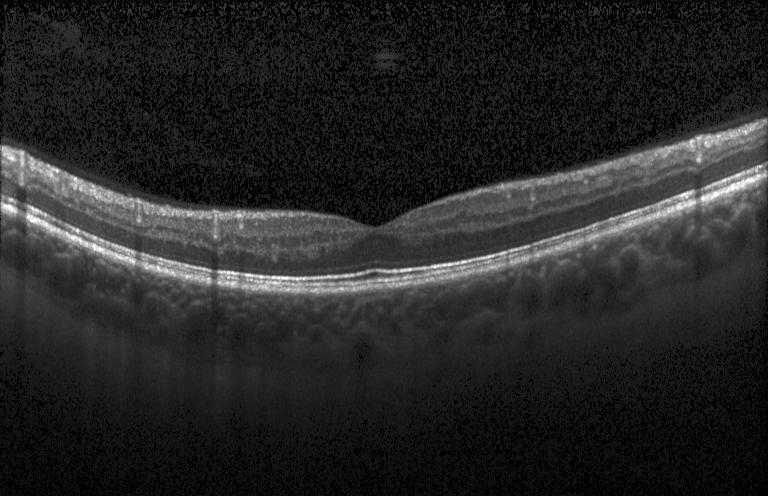

Optical coherence tomography B-scan, Heidelberg Spectralis, fovea-centered. Dx: no evidence of choroidal neovascularization, diabetic macular edema, or drusen.